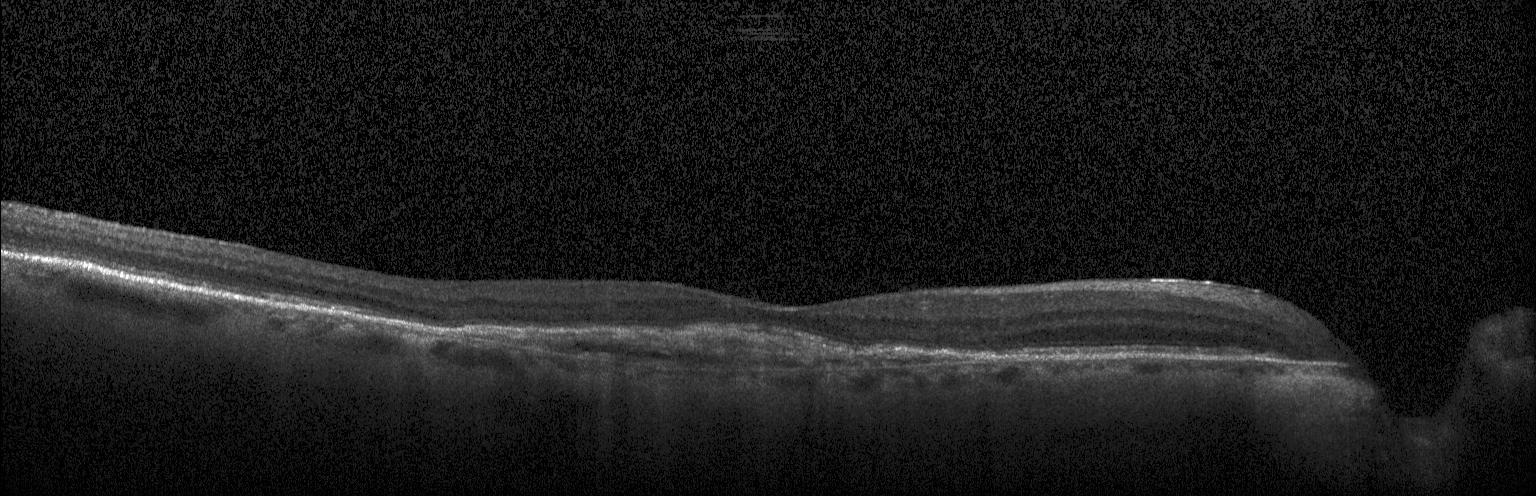 Through the macula; SD-OCT; optical coherence tomography B-scan — Assessment: CNV.